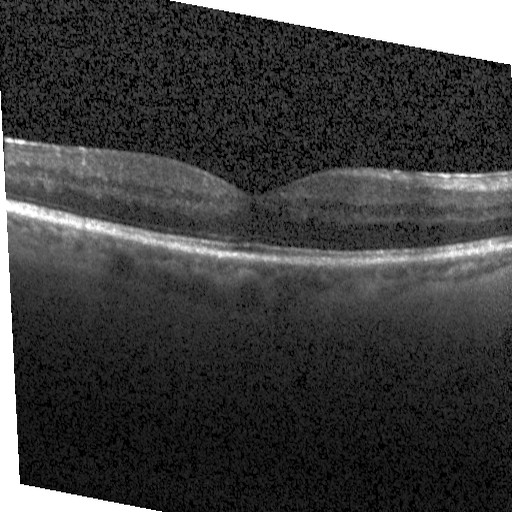 Through the macula, optical coherence tomography scan.
OCT finding: diabetic macular edema (DME).